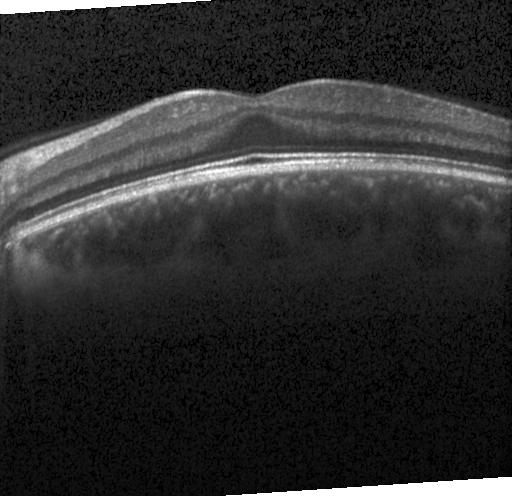
Optical coherence tomography scan. Assessment: no CNV, DME, or drusen.